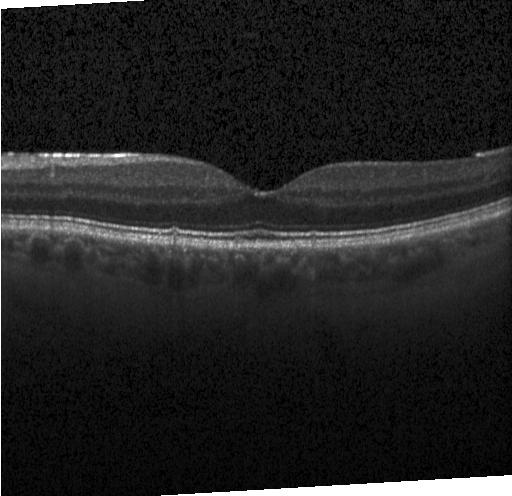
Acquired on a Heidelberg Spectralis. OCT B-scan. SD-OCT. Macular scan.
Diagnosis: neither CNV, DME, nor drusen.